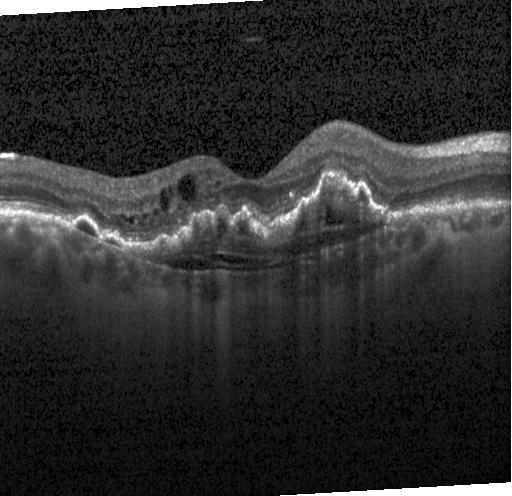
Retinal OCT cross-section showing choroidal neovascularization.